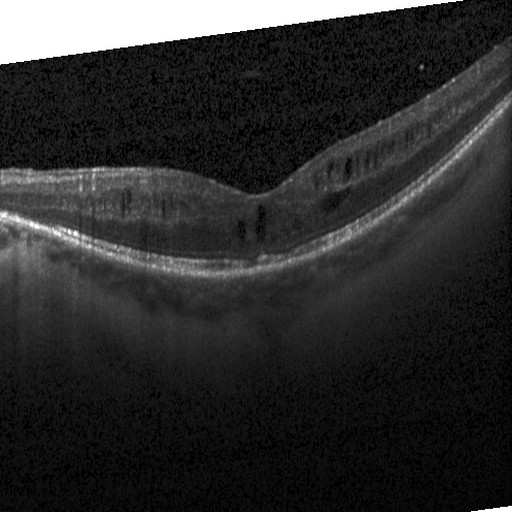
Heidelberg Spectralis OCT system; retinal OCT B-scan
The scan shows diabetic macular edema.